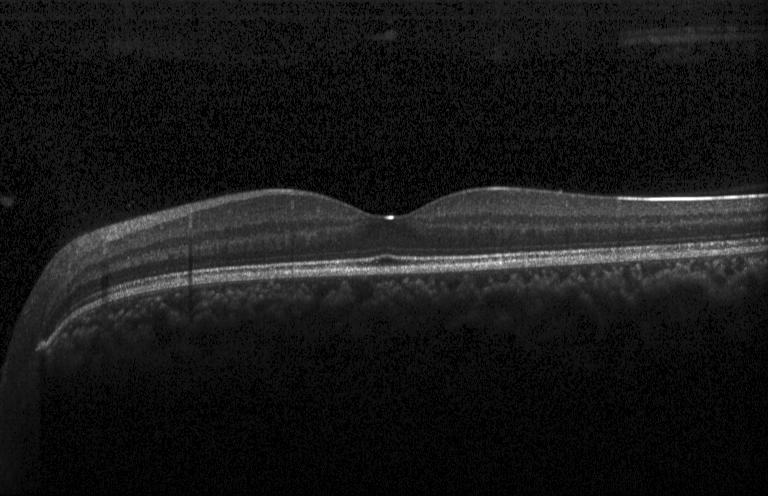
Impression: no choroidal neovascularization, no diabetic macular edema, and no drusen.